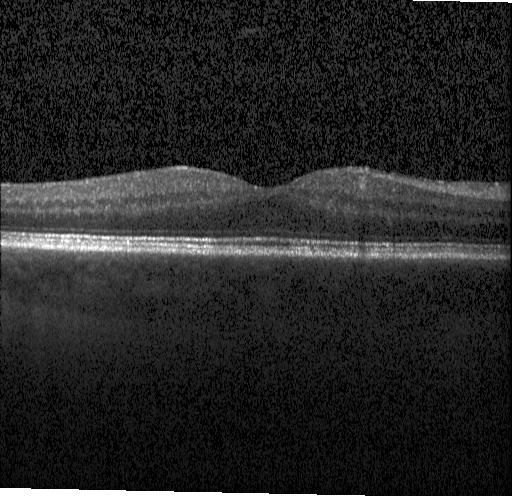 SD-OCT, acquired on a Heidelberg Spectralis, OCT B-scan
Dx: no choroidal neovascularization, no diabetic macular edema, and no drusen.